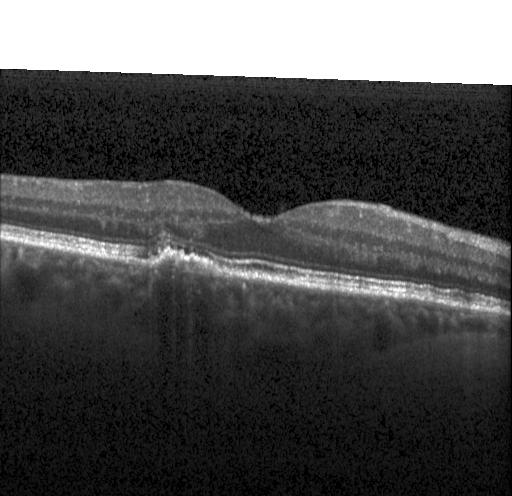 OCT finding: sub-RPE drusenoid deposits.